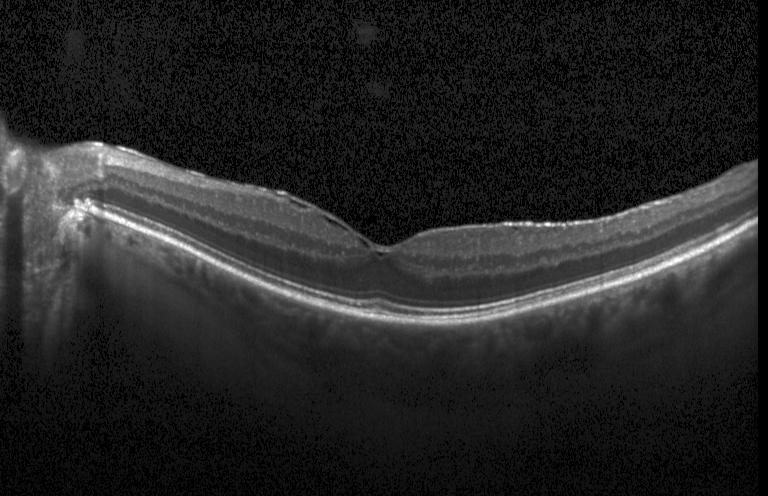
Optical coherence tomography B-scan. Impression: neither choroidal neovascularization, diabetic macular edema, nor drusen.